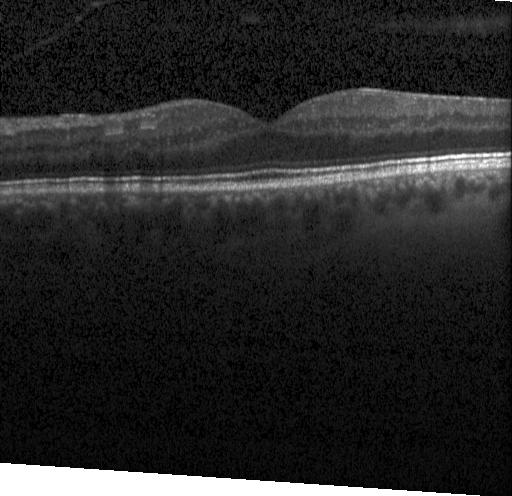

Acquired on a Heidelberg Spectralis. OCT line scan
OCT finding: neither CNV, DME, nor drusen.